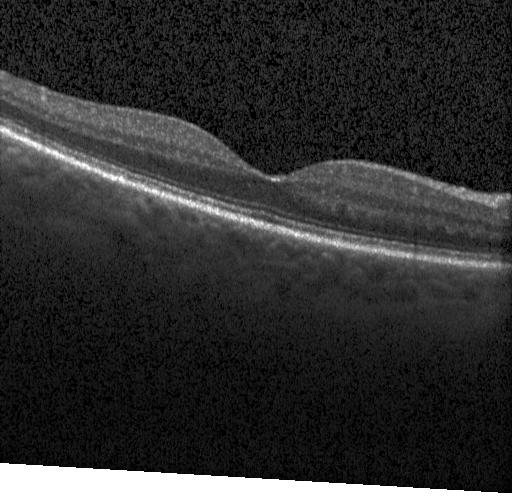

Impression: neither CNV, DME, nor drusen.